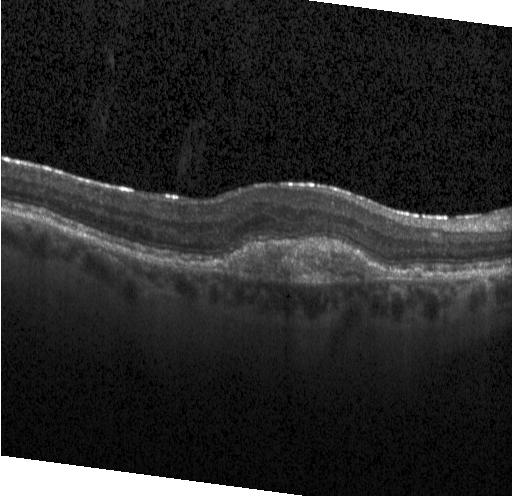

Finding: choroidal neovascularization (CNV).